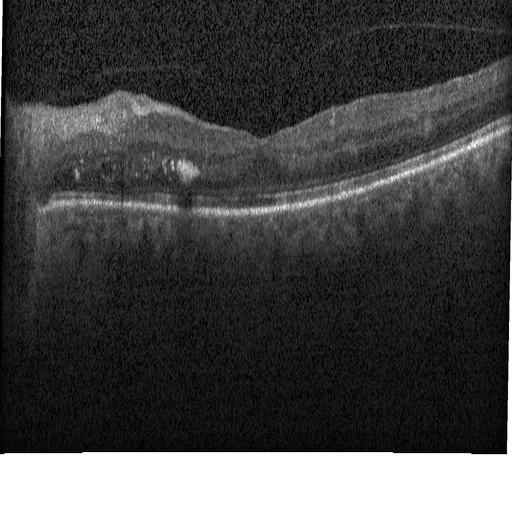 Through the macula, retinal OCT cross-section.
Diagnosis: diabetic macular edema.